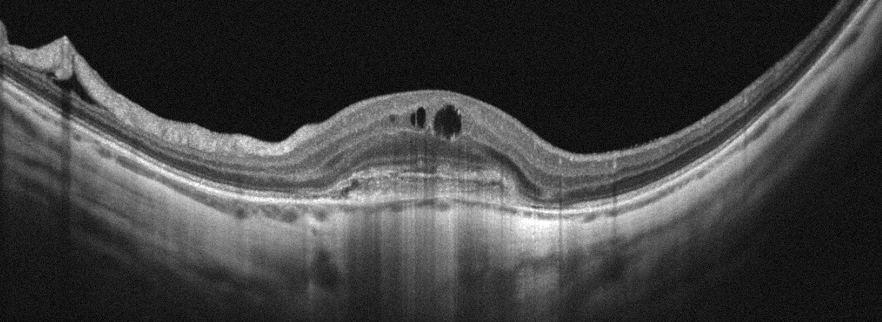 Impression: AMD.